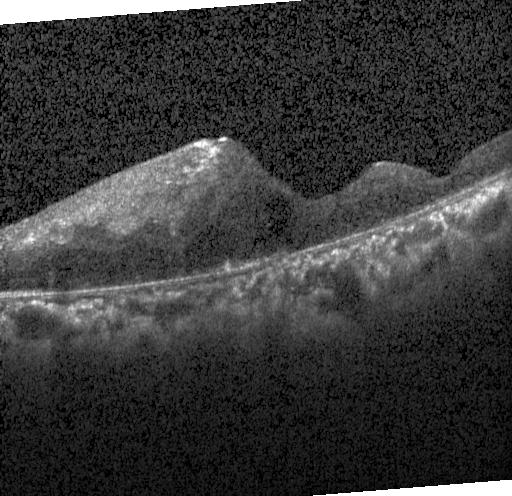

Instrument: Heidelberg Spectralis, retinal OCT B-scan, SD-OCT.
Impression: choroidal neovascularization.